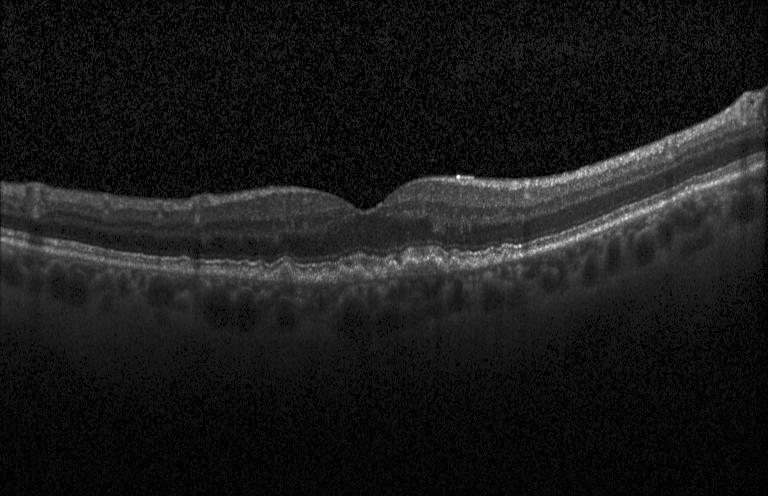
Through the macula · retinal OCT cross-section · SD-OCT · Heidelberg Spectralis OCT system.
Dx: multiple drusen.